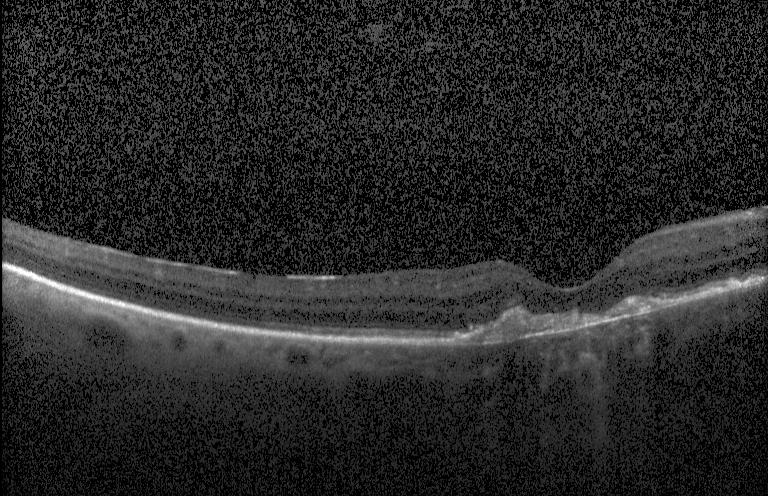
Optical coherence tomography scan; acquired on a Heidelberg Spectralis; fovea-centered; spectral-domain OCT.
Diagnosis: CNV.